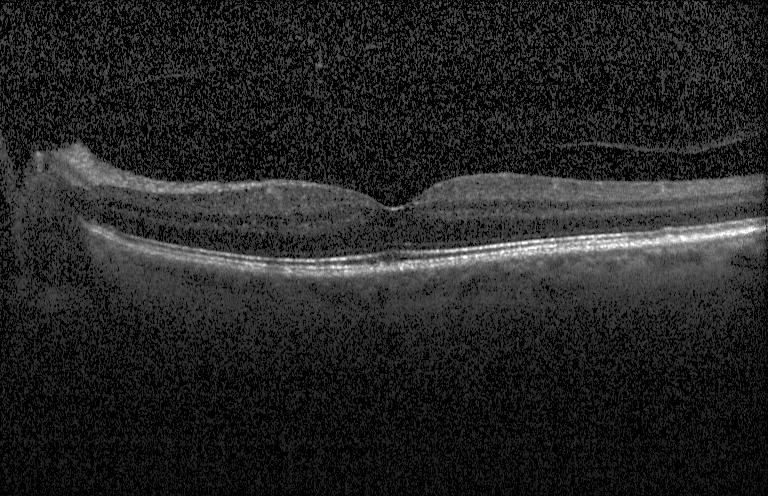 Retinal OCT B-scan, through the macula, SD-OCT. Impression: no CNV, no DME, and no drusen.